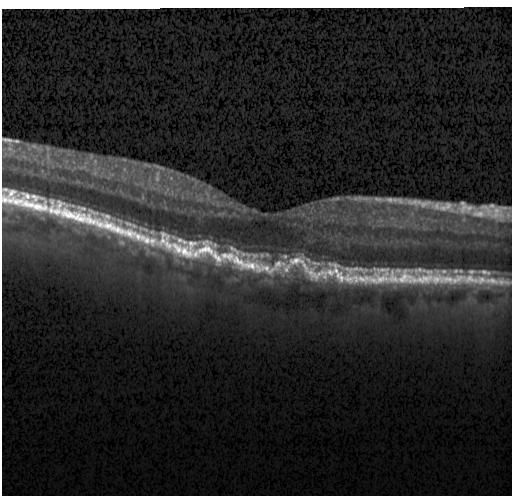
SD-OCT, centered on the fovea, Heidelberg Spectralis OCT system, retinal OCT B-scan. Assessment: multiple drusen.